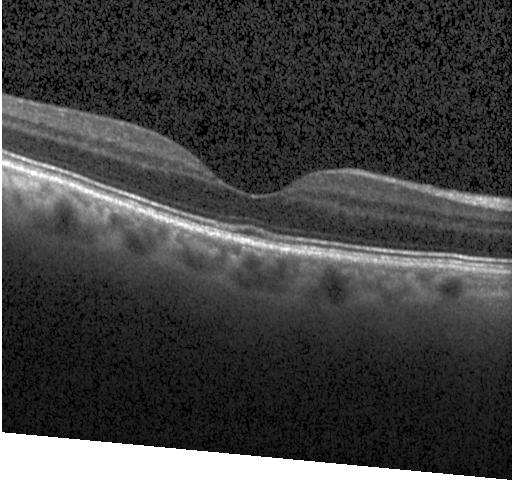
Retinal OCT cross-section.
Diagnosis: no choroidal neovascularization, no diabetic macular edema, and no drusen.